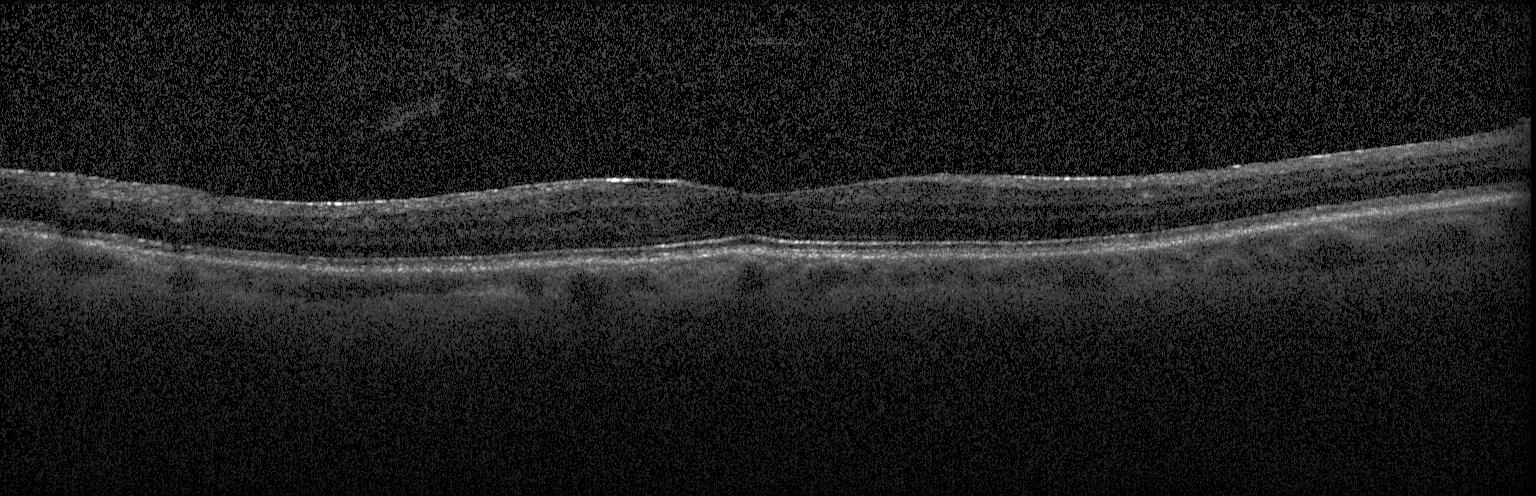
Optical coherence tomography scan; spectral-domain optical coherence tomography. Dx: neither choroidal neovascularization, diabetic macular edema, nor drusen.